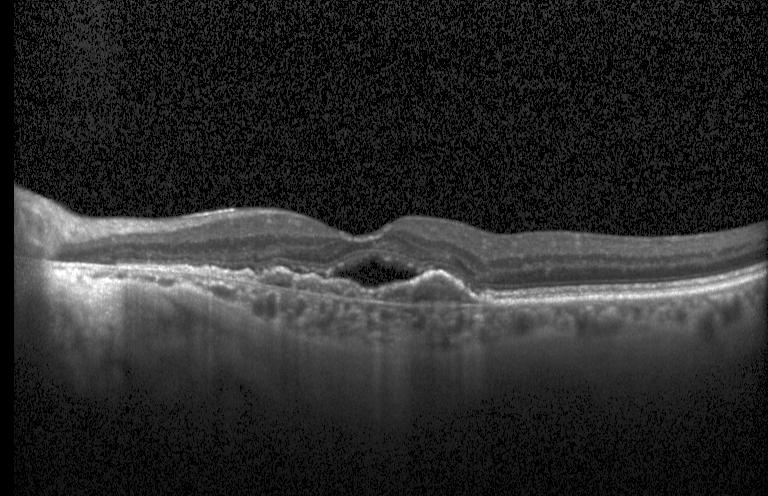
Spectral-domain OCT · centered on the fovea · optical coherence tomography scan.
Assessment: CNV.